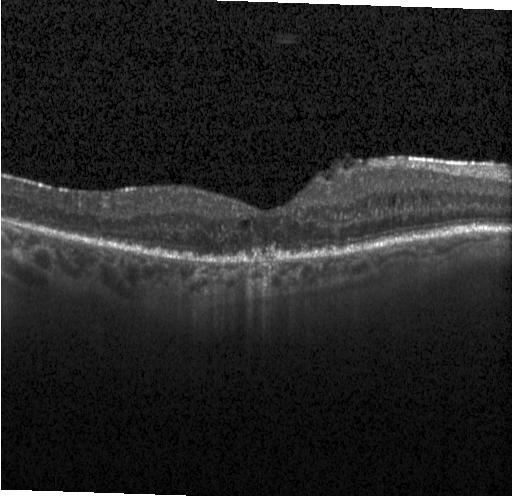 Retinal OCT cross-section — Finding: no evidence of choroidal neovascularization, diabetic macular edema, or drusen.